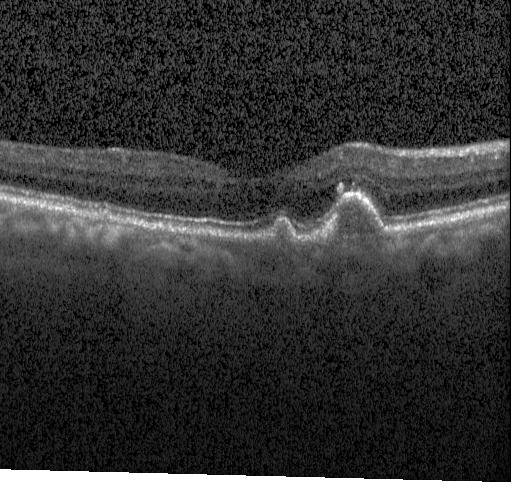 Dx: drusen.